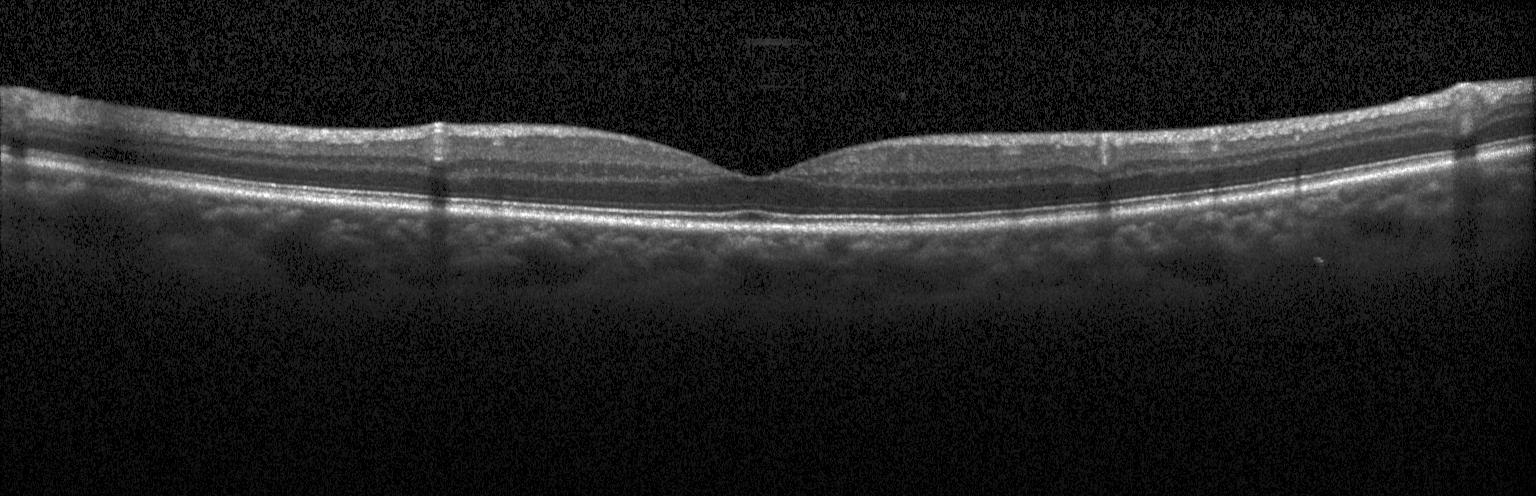 Macular OCT demonstrating no CNV, no DME, and no drusen.